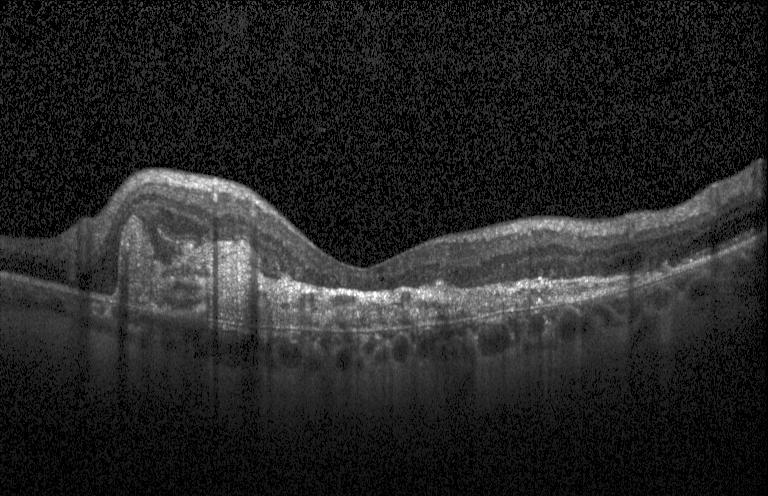

Impression: a choroidal neovascular membrane.